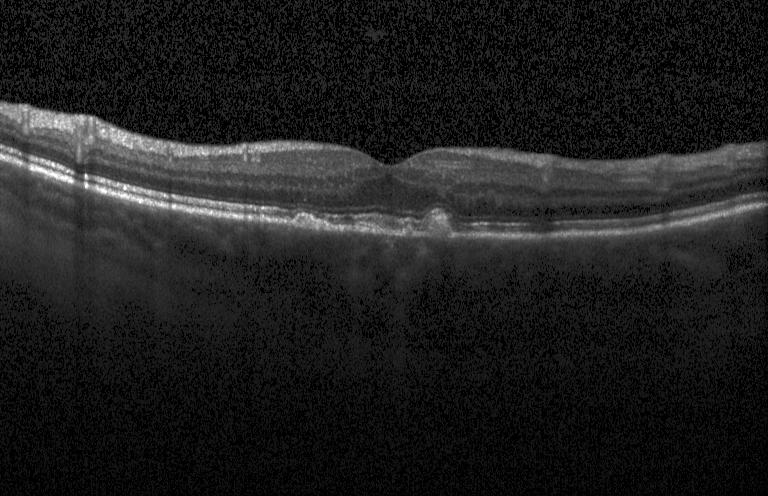
Dx: drusen.